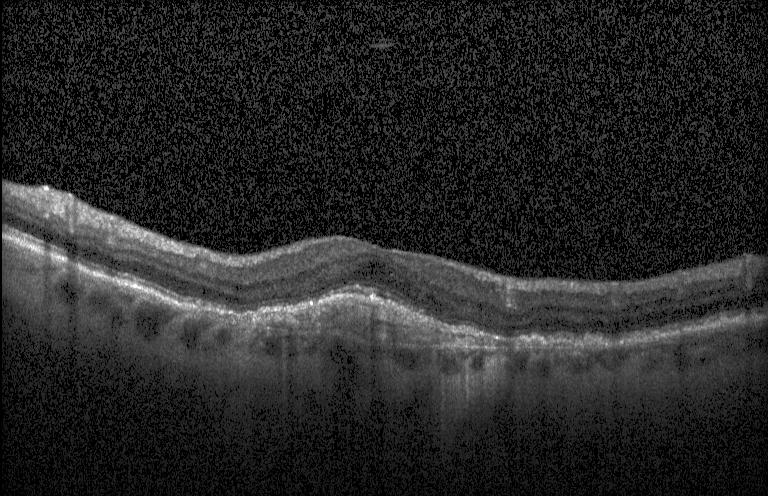 OCT line scan.
Diagnosis: CNV.